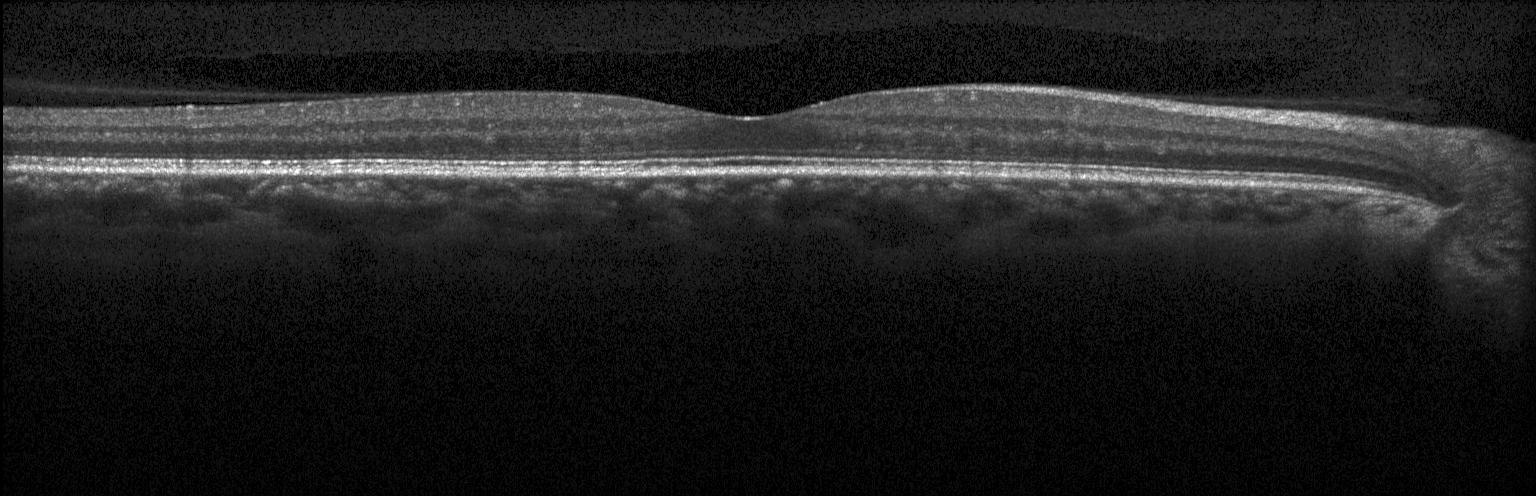

OCT B-scan; Heidelberg Spectralis OCT system. Diagnosis: no CNV, no DME, and no drusen.